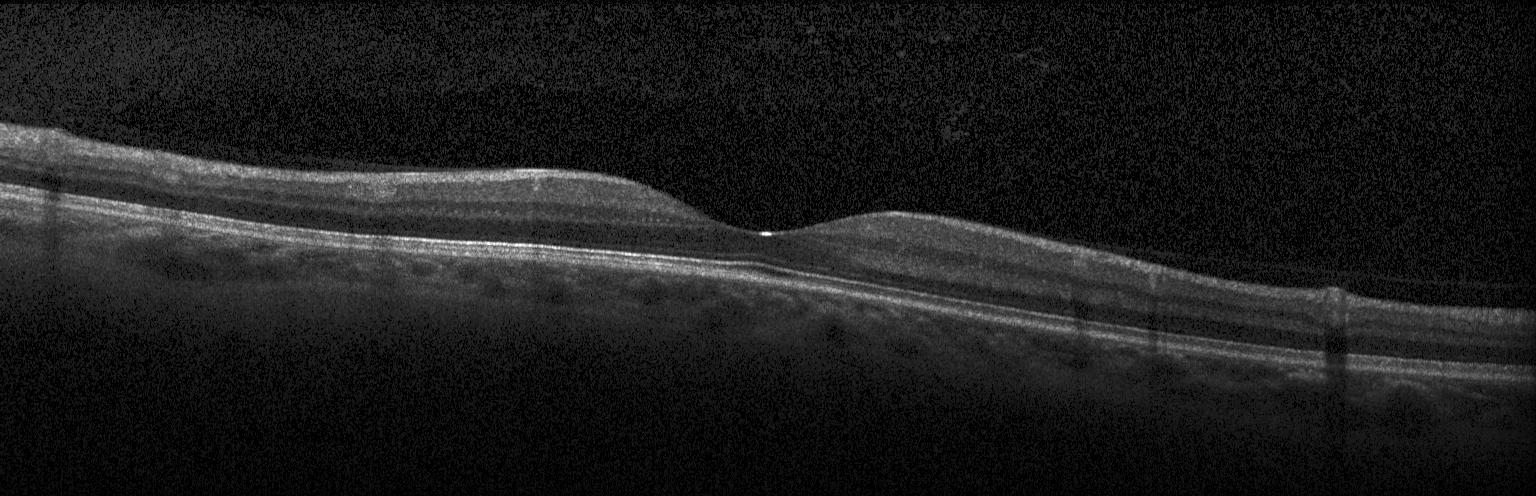
Spectral-domain OCT B-scan: no CNV, DME, or drusen.